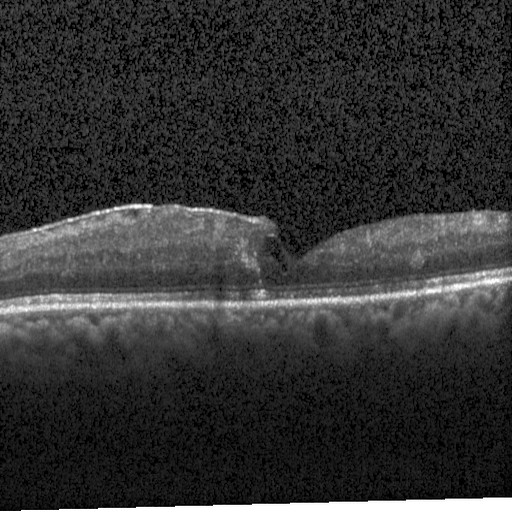 Fovea-centered; optical coherence tomography B-scan
Diagnosis: DME.